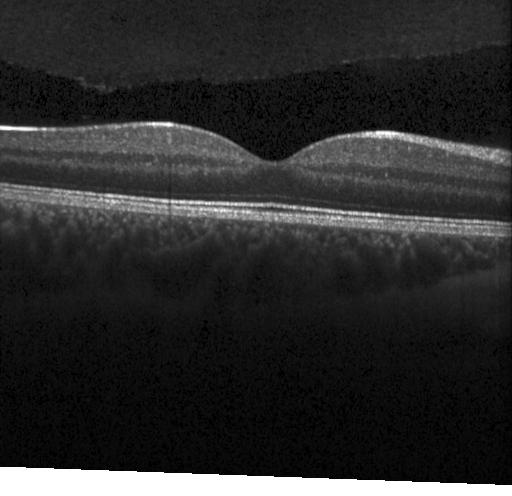
Optical coherence tomography B-scan. Finding: neither CNV, DME, nor drusen.